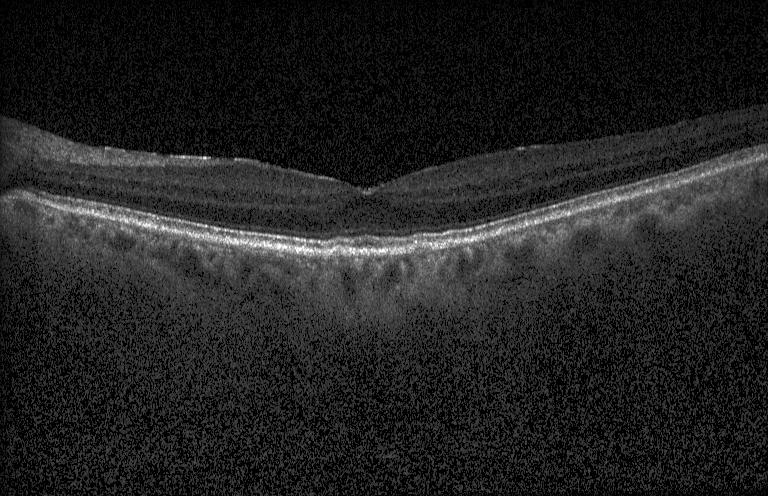 OCT line scan. This B-scan demonstrates drusen.